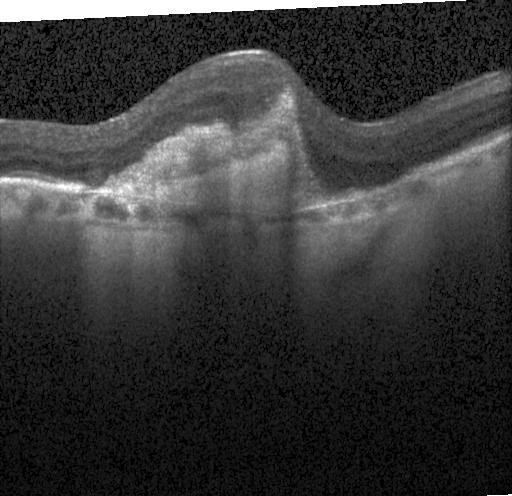

Retinal OCT B-scan — Diagnosis: a choroidal neovascular membrane.